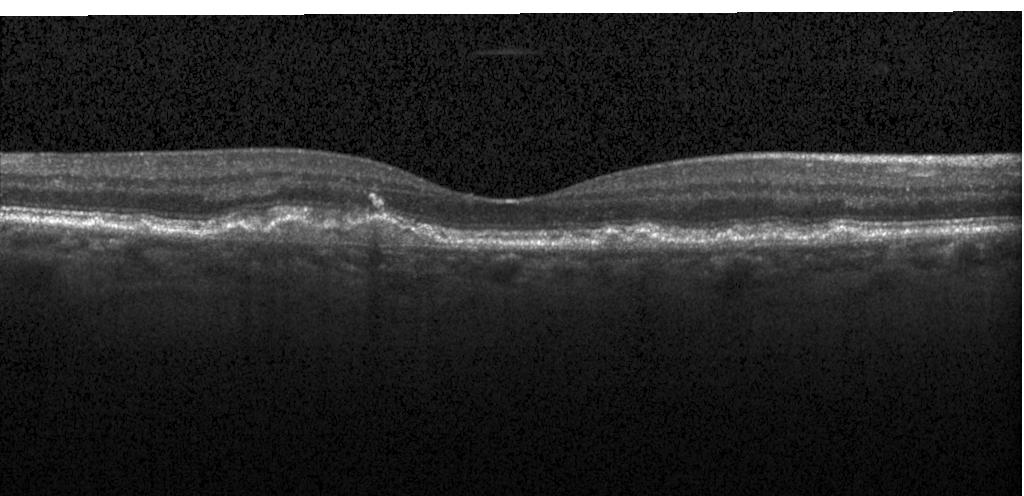
Dx: a choroidal neovascular membrane.